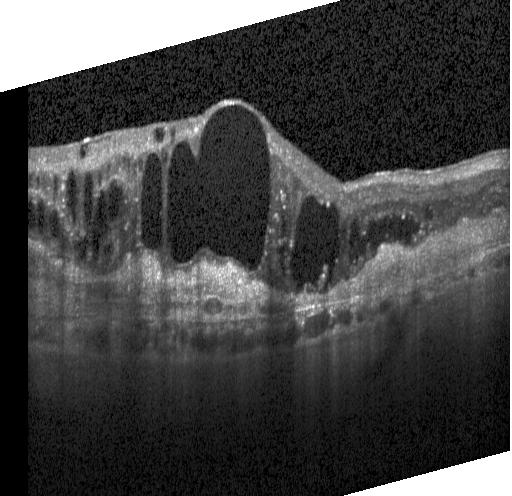 OCT B-scan showing a choroidal neovascular membrane.